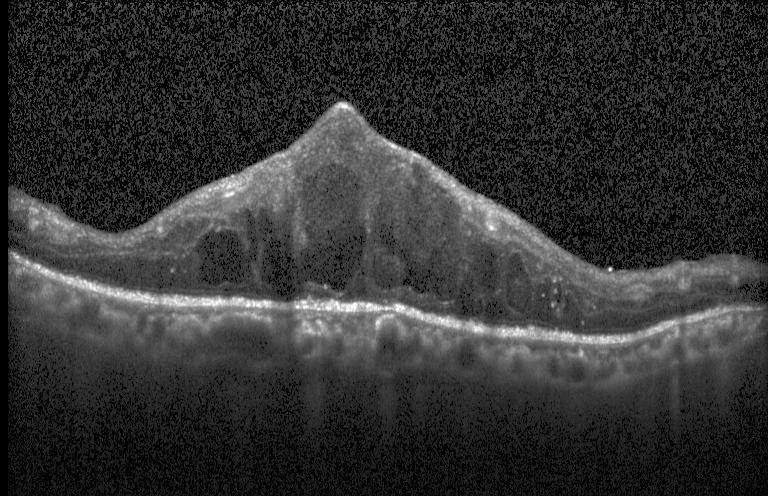 Fovea-centered · spectral-domain optical coherence tomography · optical coherence tomography scan · acquired on a Heidelberg Spectralis
Dx: diabetic macular edema.